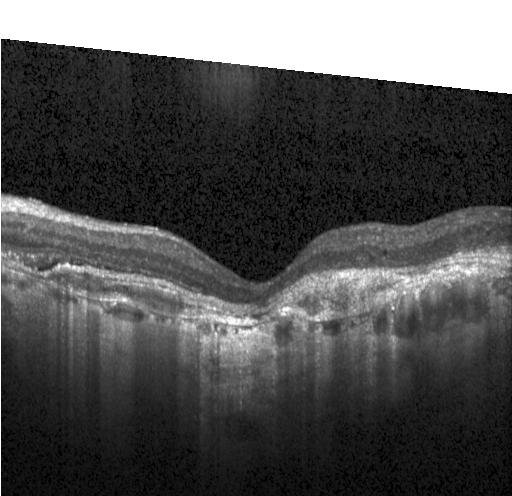 Macular OCT demonstrating a choroidal neovascular membrane.